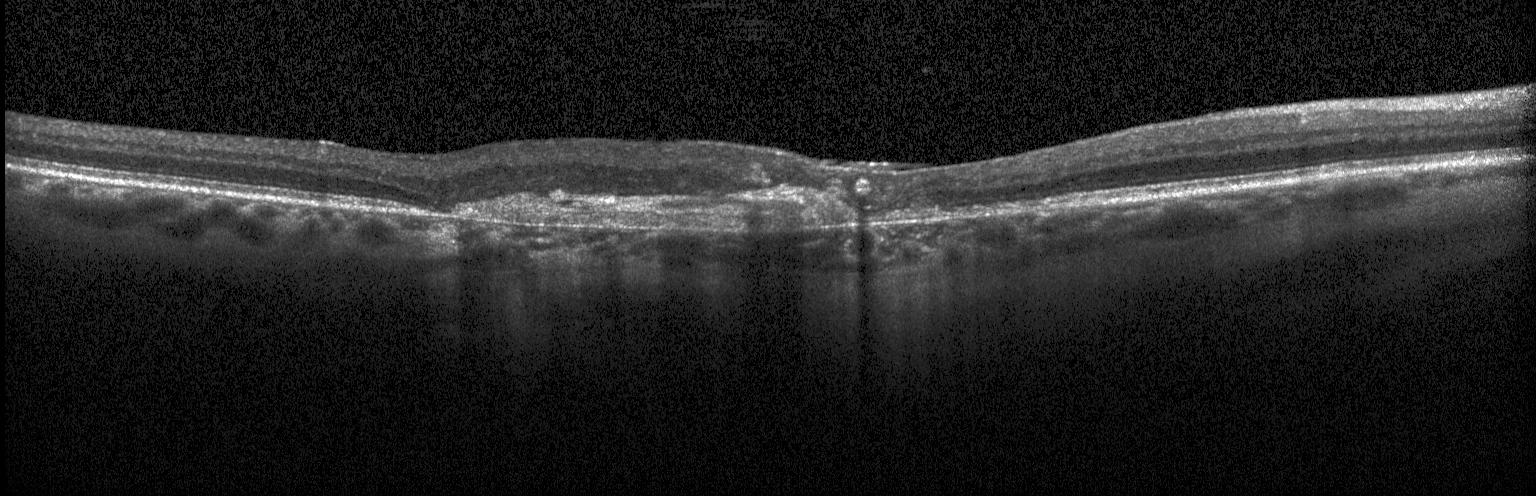
OCT line scan
Choroidal neovascularization.